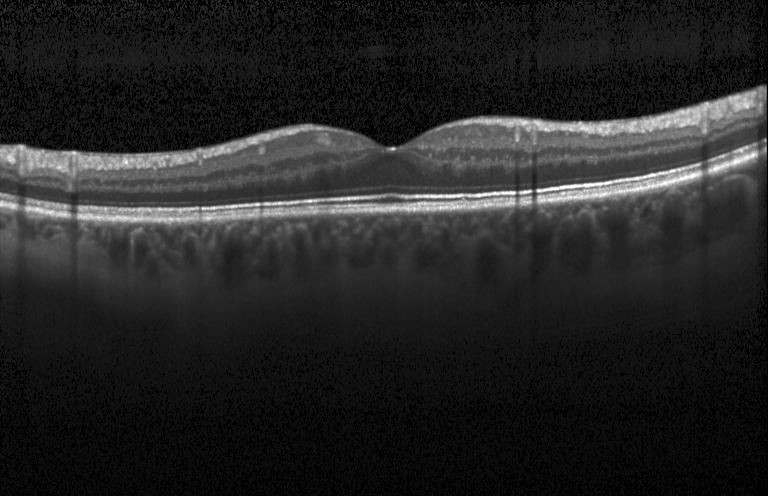
Through the macula · Heidelberg Spectralis OCT system · spectral-domain OCT · retinal OCT B-scan
Macular OCT: neither choroidal neovascularization, diabetic macular edema, nor drusen.